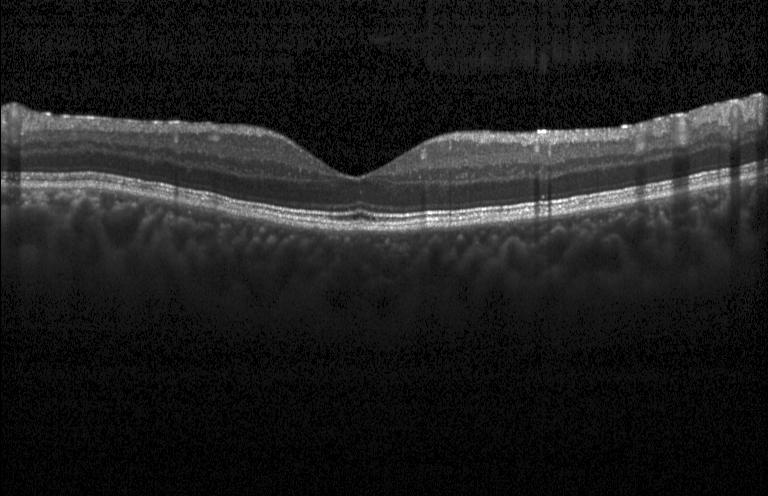 Through the macula; retinal OCT B-scan — Assessment: neither choroidal neovascularization, diabetic macular edema, nor drusen.